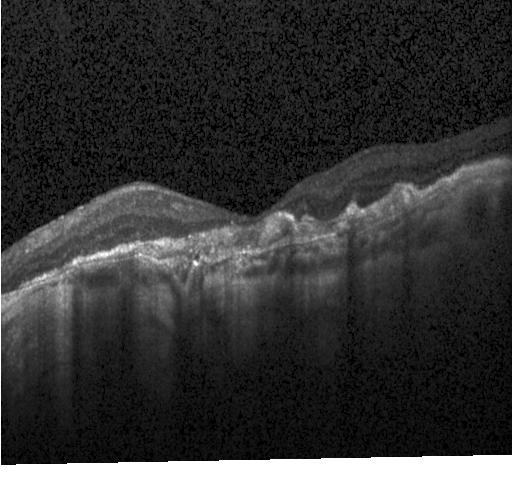 Dx: a choroidal neovascular membrane.